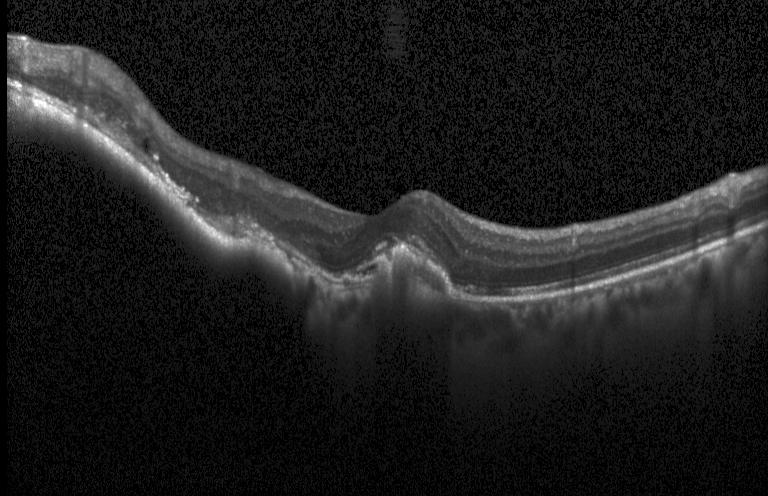 SD-OCT; retinal OCT cross-section; through the macula. Dx: a choroidal neovascular membrane.